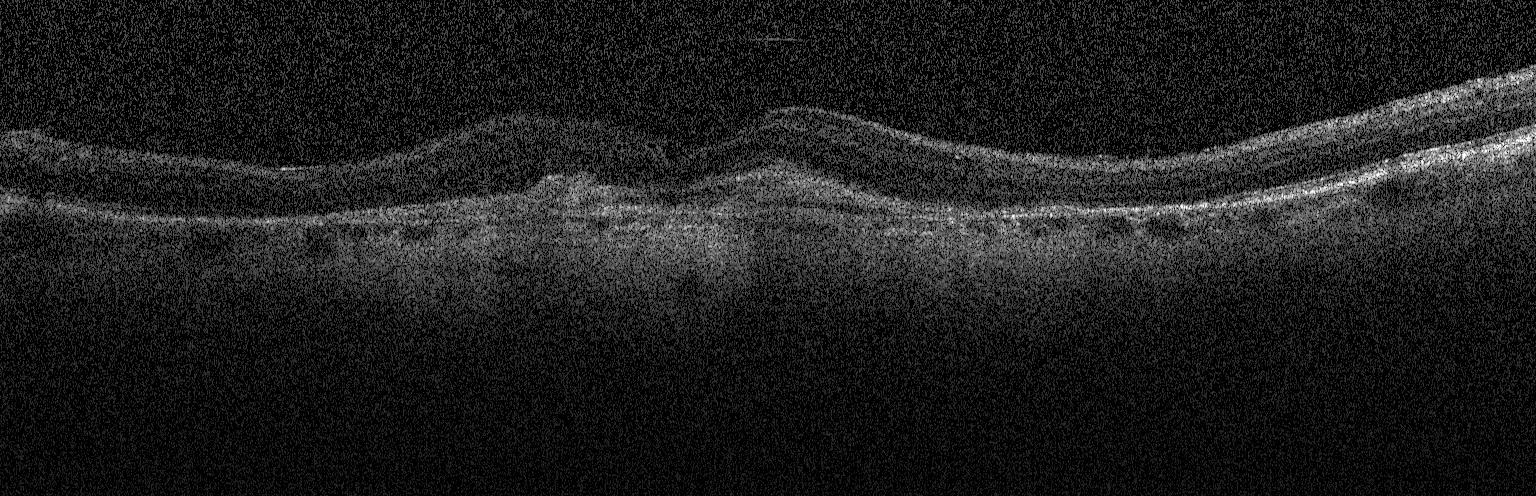

Optical coherence tomography B-scan. Through the macula — Macular OCT: CNV.